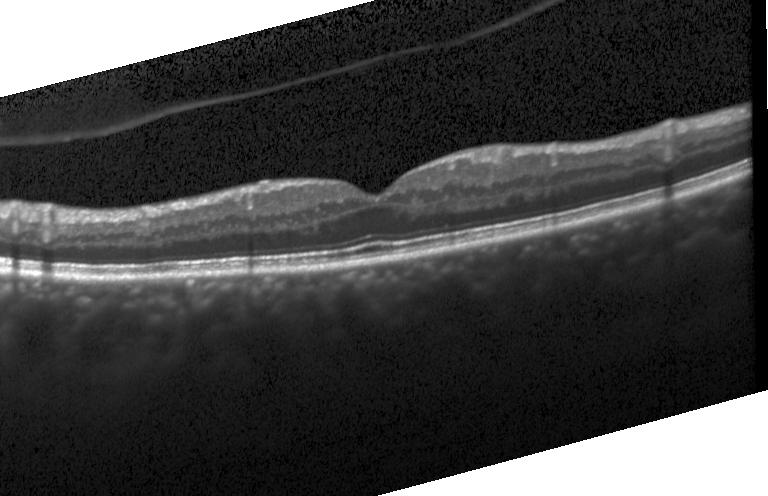 Through the macula, retinal OCT B-scan.
Diagnosis: no evidence of choroidal neovascularization, diabetic macular edema, or drusen.